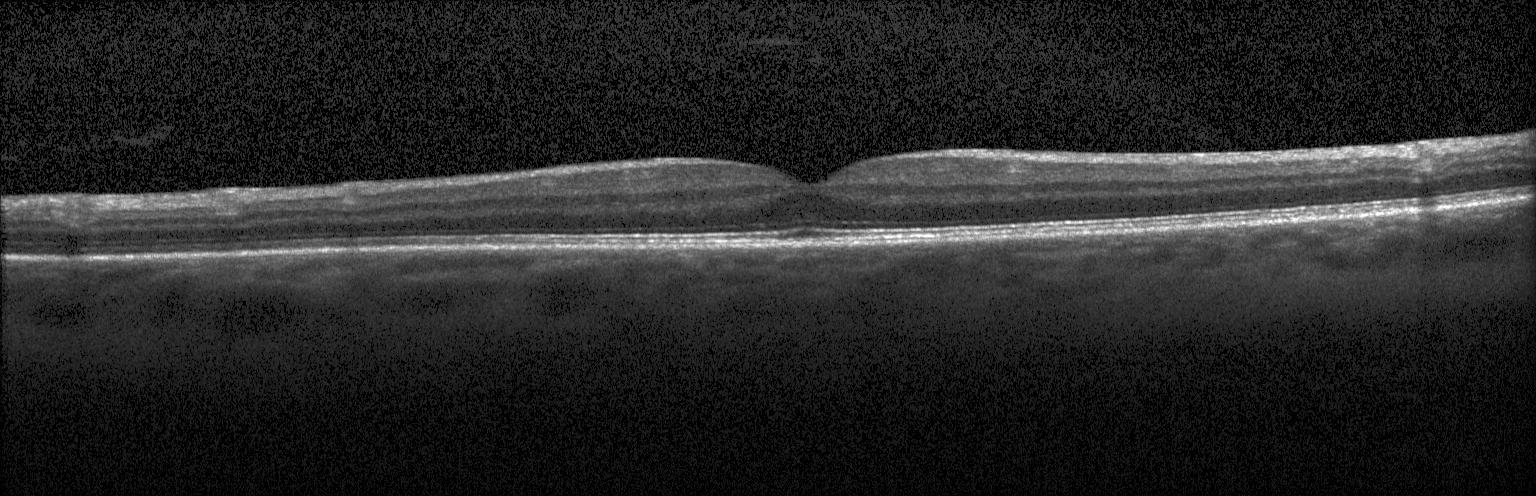
Optical coherence tomography B-scan, spectral-domain OCT, instrument: Heidelberg Spectralis.
Assessment: no choroidal neovascularization, diabetic macular edema, or drusen.